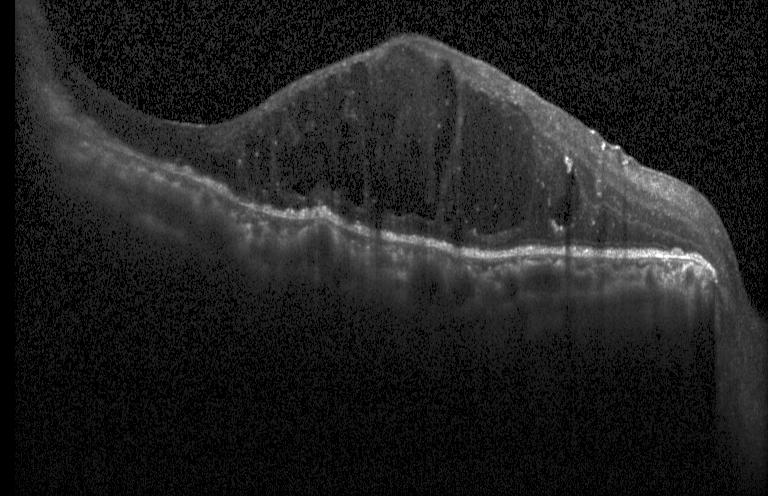
Diagnosis: DME.